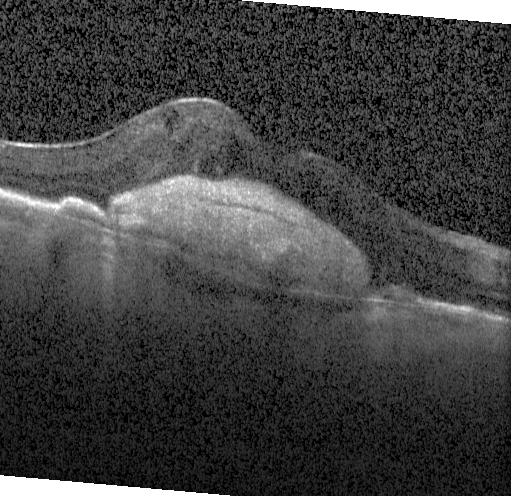 Diagnosis: CNV.